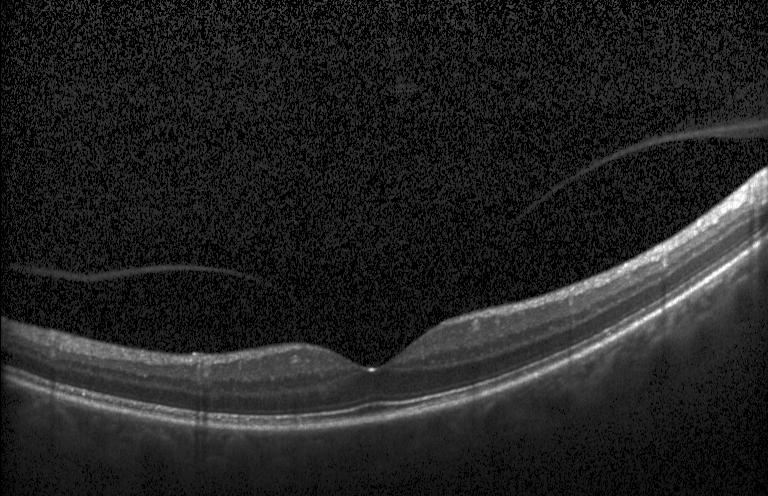
Finding: no choroidal neovascularization, diabetic macular edema, or drusen.